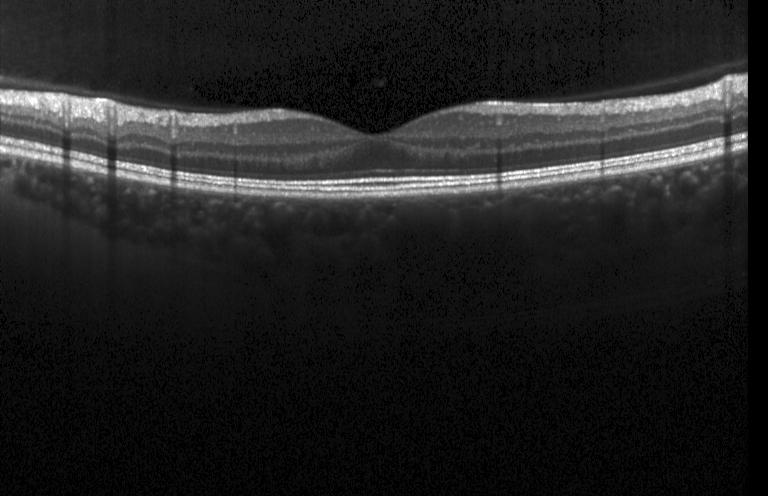

Optical coherence tomography scan, spectral-domain OCT, fovea-centered, Heidelberg Spectralis OCT system
This B-scan demonstrates no evidence of CNV, DME, or drusen.